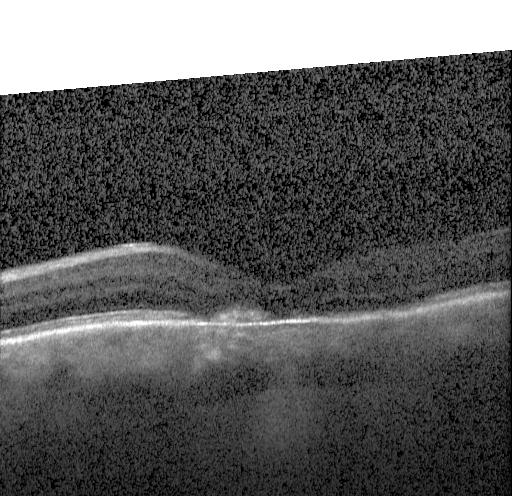 Retinal OCT cross-section. SD-OCT.
This B-scan demonstrates a choroidal neovascular membrane.